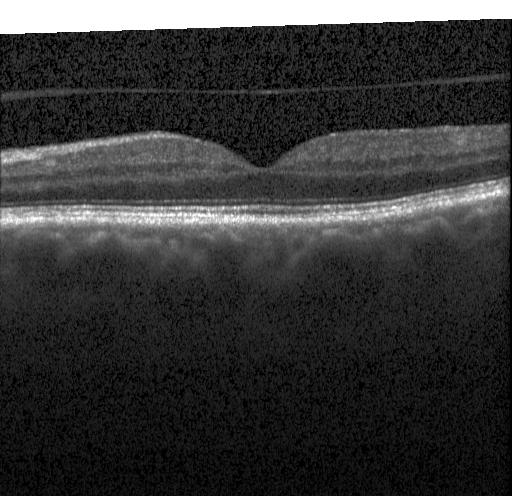
OCT B-scan showing no choroidal neovascularization, diabetic macular edema, or drusen.